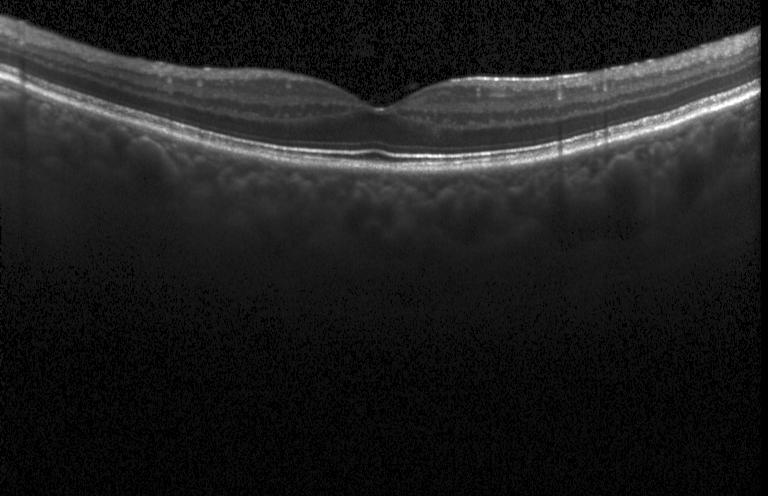
Impression: no choroidal neovascularization, no diabetic macular edema, and no drusen.